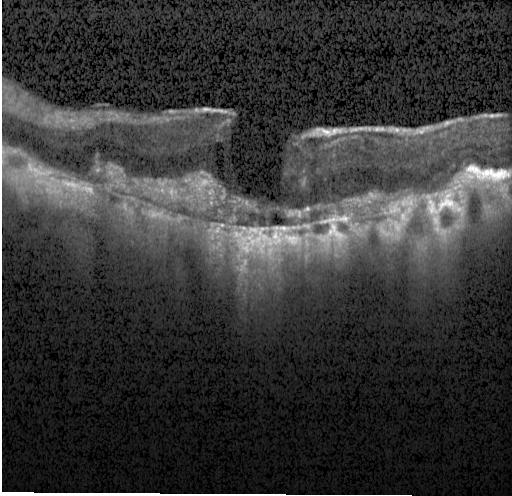
OCT B-scan, spectral-domain OCT — Dx: CNV.